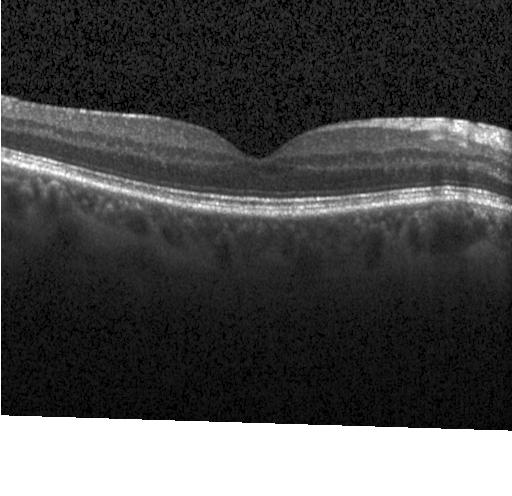

Optical coherence tomography B-scan. Finding: neither CNV, DME, nor drusen.